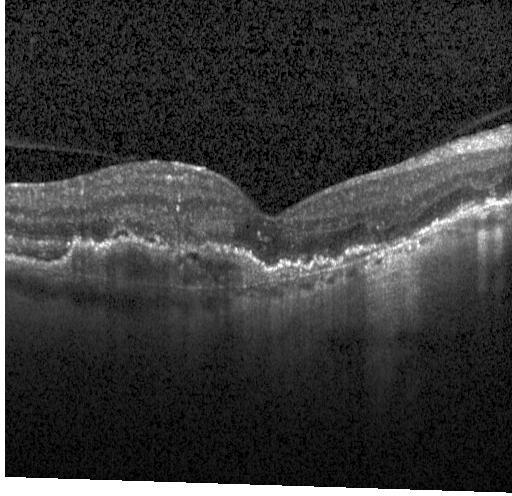
Macular OCT: choroidal neovascularization.